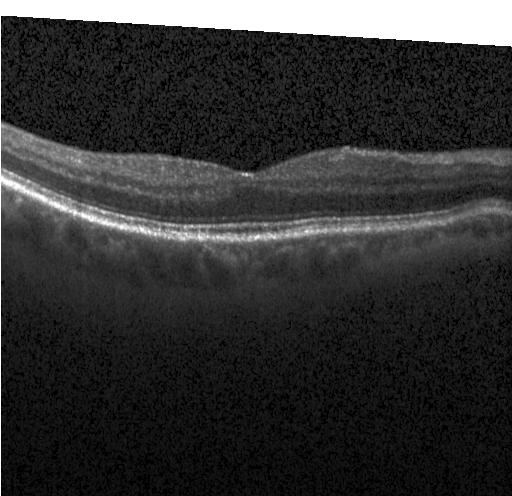 Optical coherence tomography B-scan. OCT finding: neither choroidal neovascularization, diabetic macular edema, nor drusen.